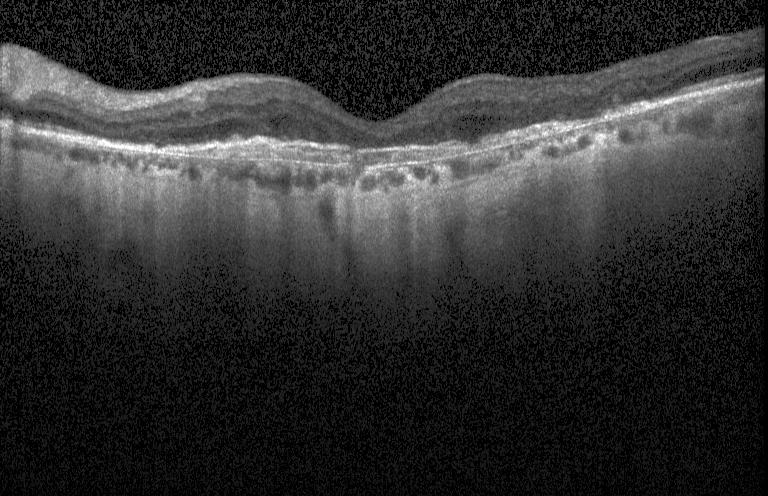 Centered on the fovea · spectral-domain OCT · Heidelberg Spectralis OCT system · OCT line scan — Impression: a choroidal neovascular membrane.